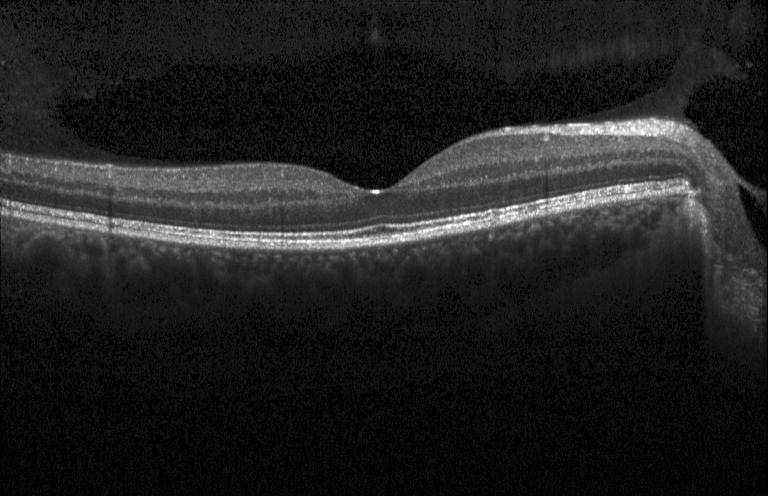
Spectral-domain OCT. OCT B-scan
OCT finding: neither choroidal neovascularization, diabetic macular edema, nor drusen.